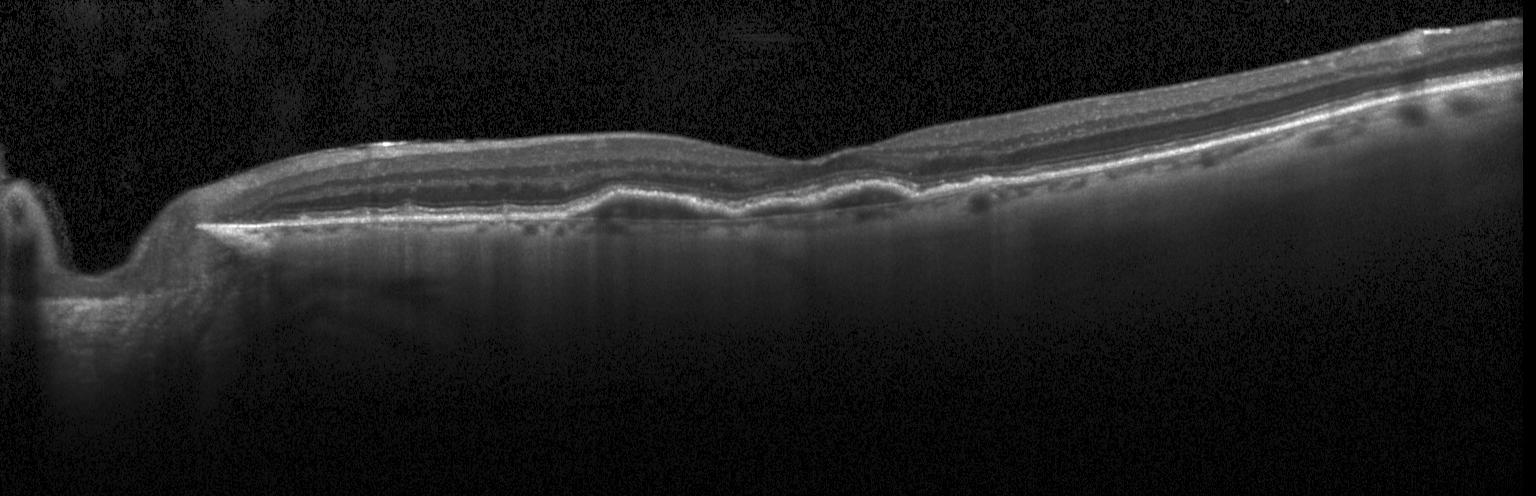
Through the macula, optical coherence tomography B-scan, spectral-domain OCT — Assessment: choroidal neovascularization (CNV).